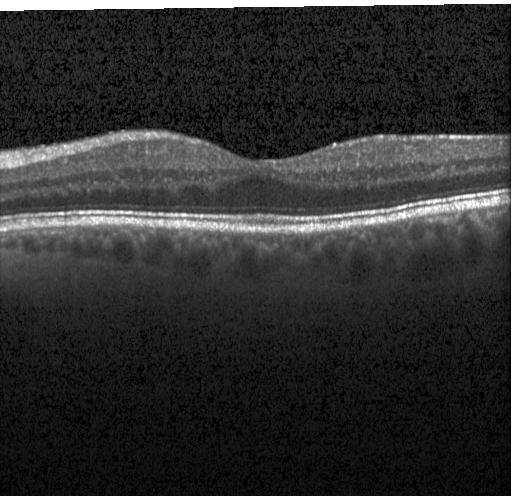
OCT B-scan
Impression: no CNV, DME, or drusen.